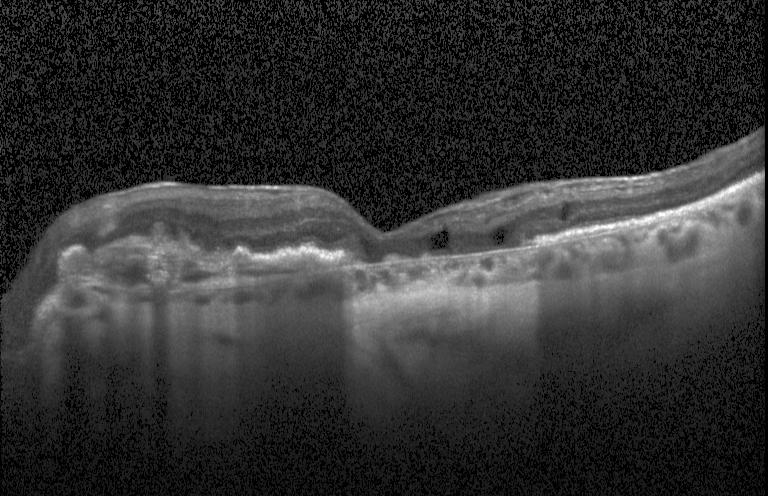
Optical coherence tomography B-scan.
This B-scan demonstrates CNV.